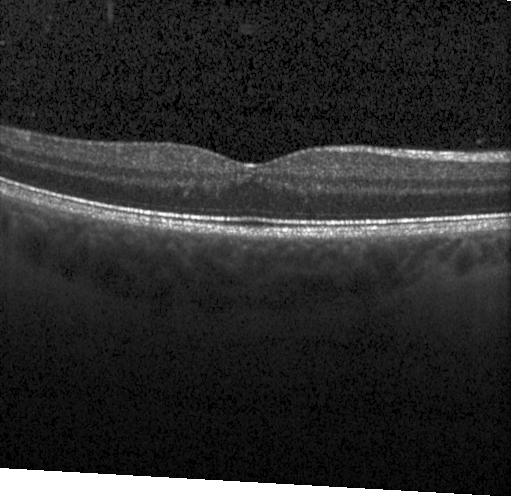

Optical coherence tomography scan · horizontal scan through the fovea · Heidelberg Spectralis.
Assessment: no CNV, DME, or drusen.